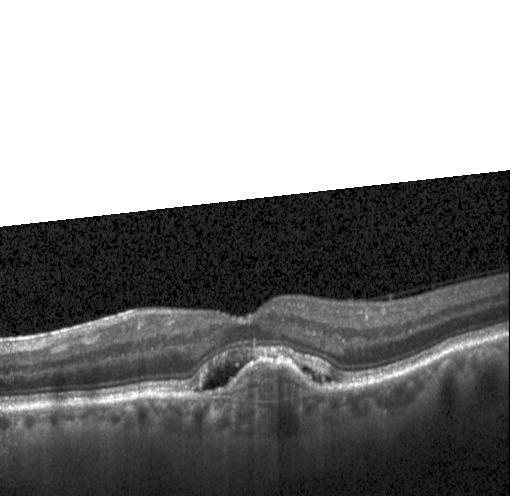 Retinal OCT cross-section, Heidelberg Spectralis OCT system. Assessment: a choroidal neovascular membrane.